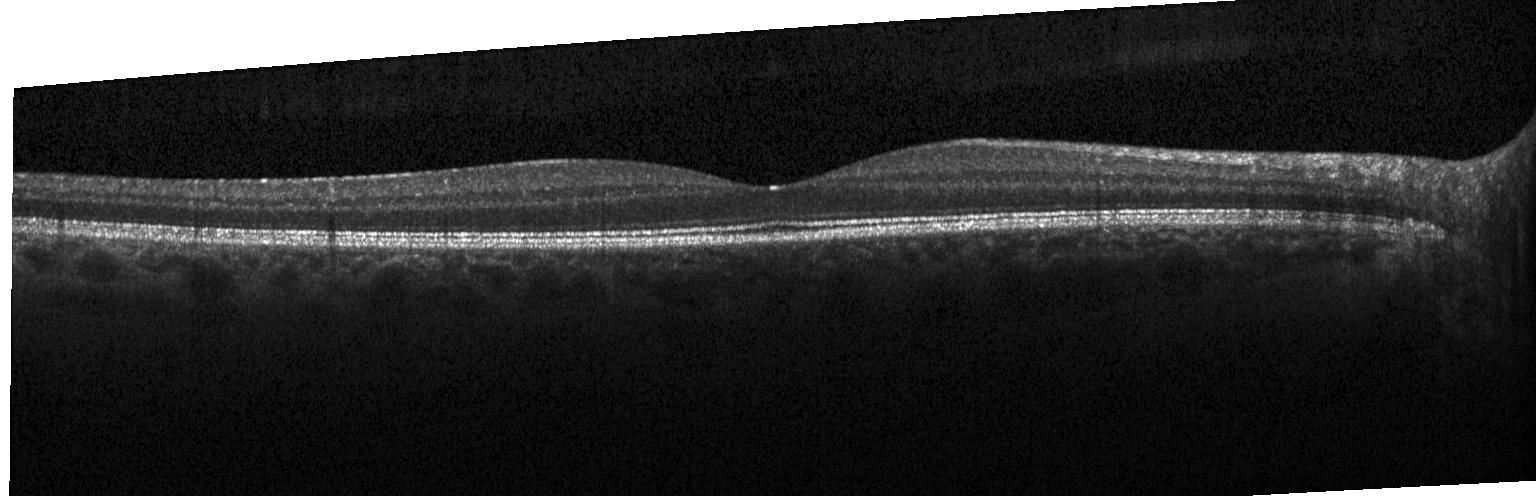

Heidelberg Spectralis OCT system · OCT B-scan. Impression: no evidence of CNV, DME, or drusen.